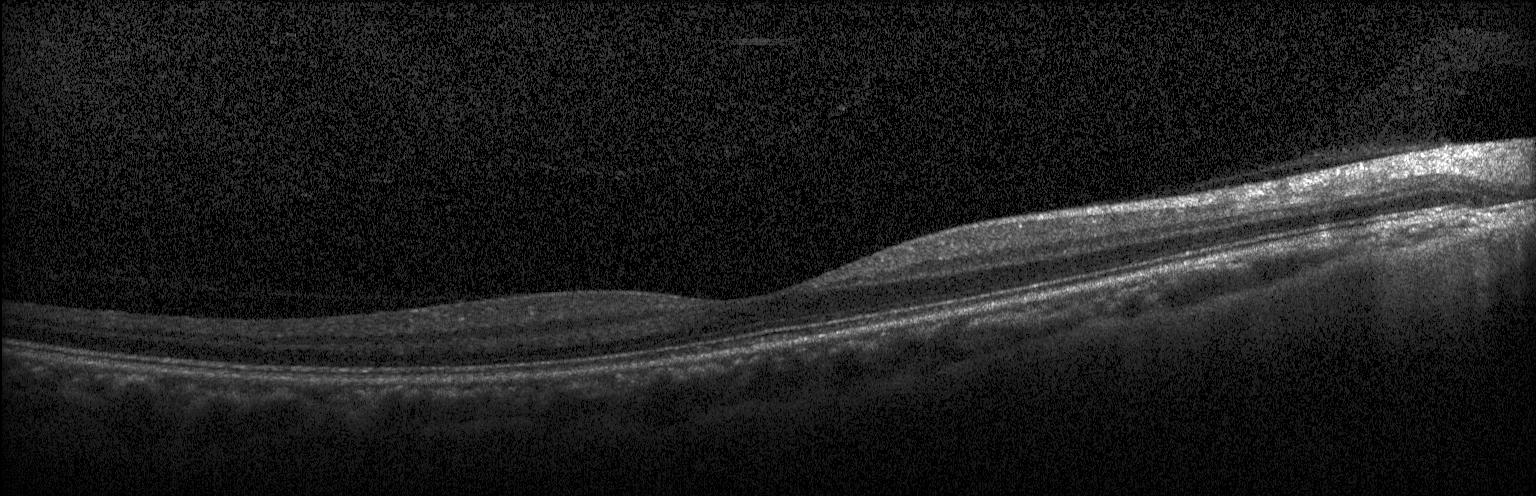 Heidelberg Spectralis OCT system · centered on the fovea · retinal OCT cross-section · spectral-domain OCT. OCT finding: no evidence of choroidal neovascularization, diabetic macular edema, or drusen.